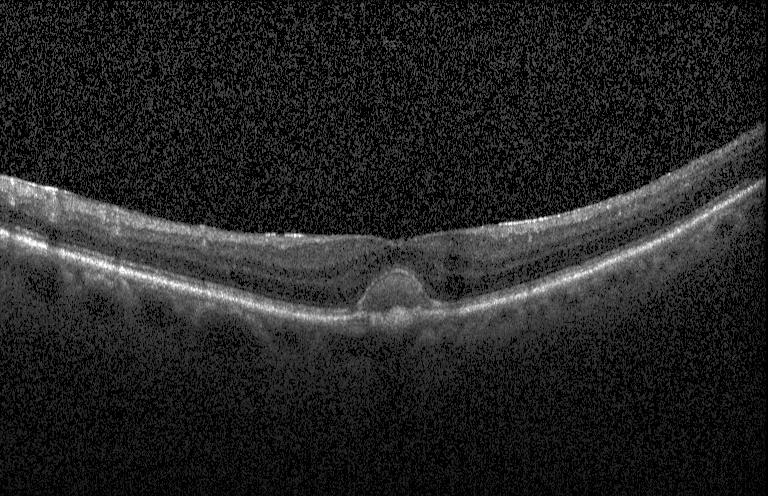

Spectral-domain OCT B-scan: a choroidal neovascular membrane.